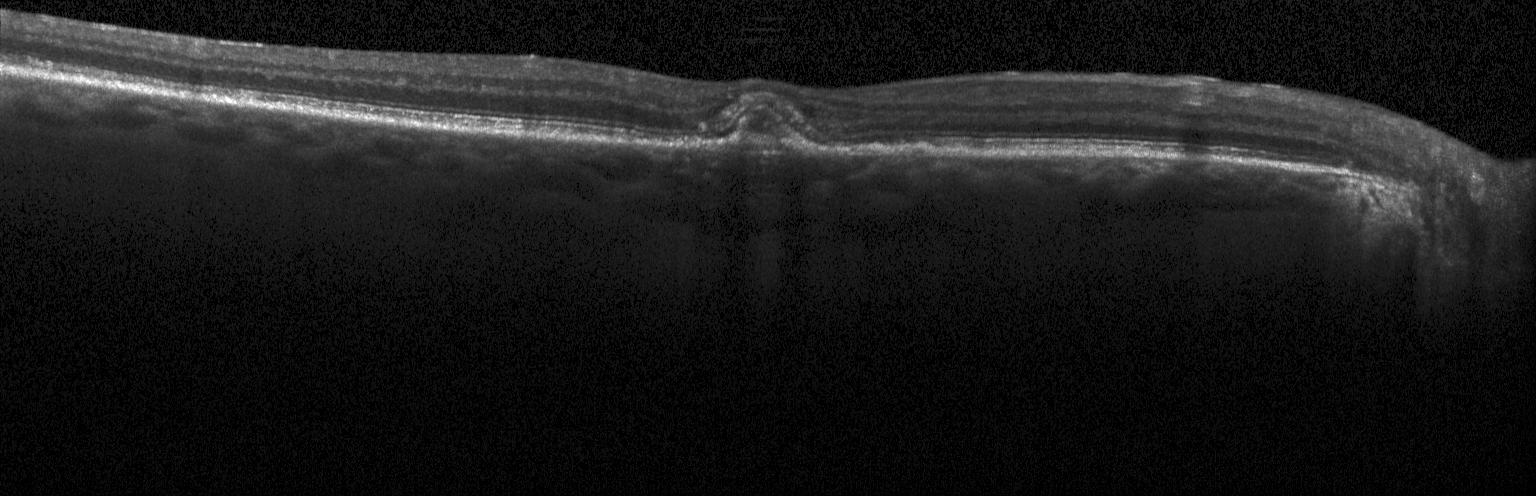 OCT B-scan. Spectral-domain optical coherence tomography — Assessment: a choroidal neovascular membrane.